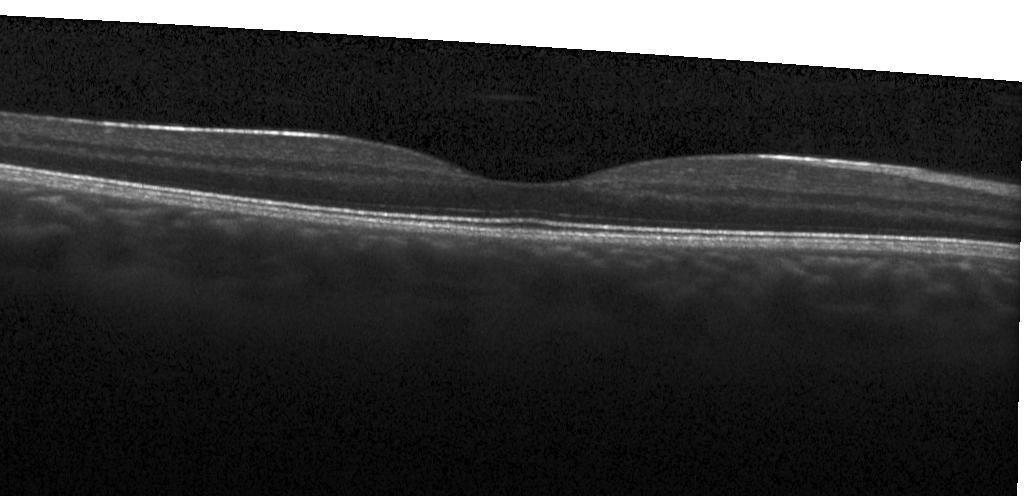

Assessment: no evidence of CNV, DME, or drusen.